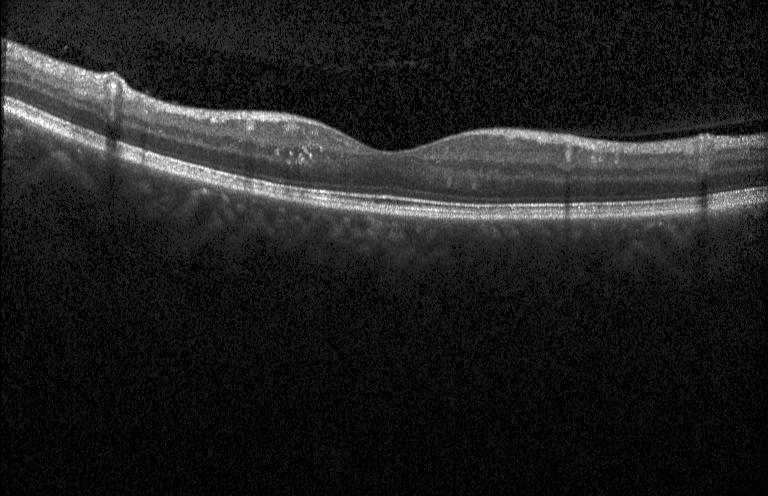
Retinal OCT B-scan
Diagnosis: neither choroidal neovascularization, diabetic macular edema, nor drusen.